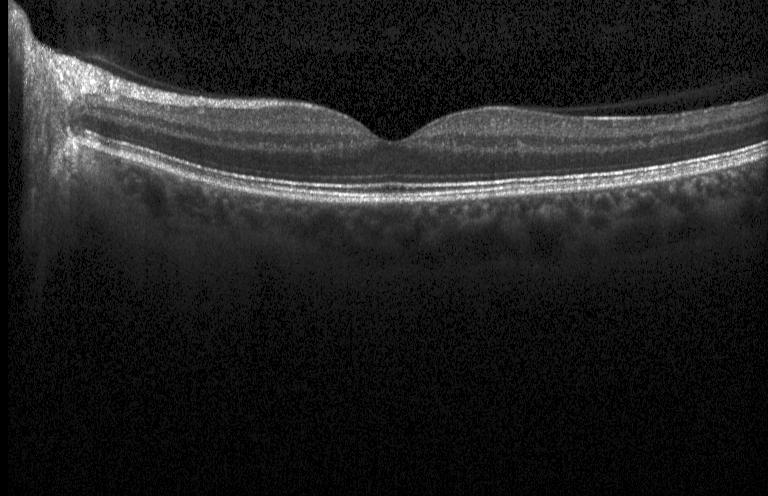

Optical coherence tomography B-scan.
This B-scan demonstrates no choroidal neovascularization, diabetic macular edema, or drusen.